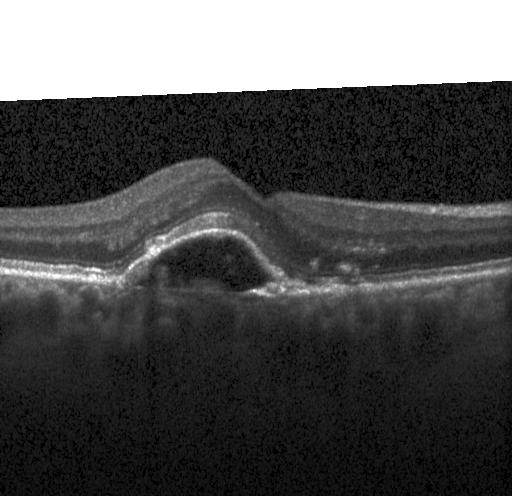 OCT line scan · spectral-domain OCT · fovea-centered — Finding: a choroidal neovascular membrane.